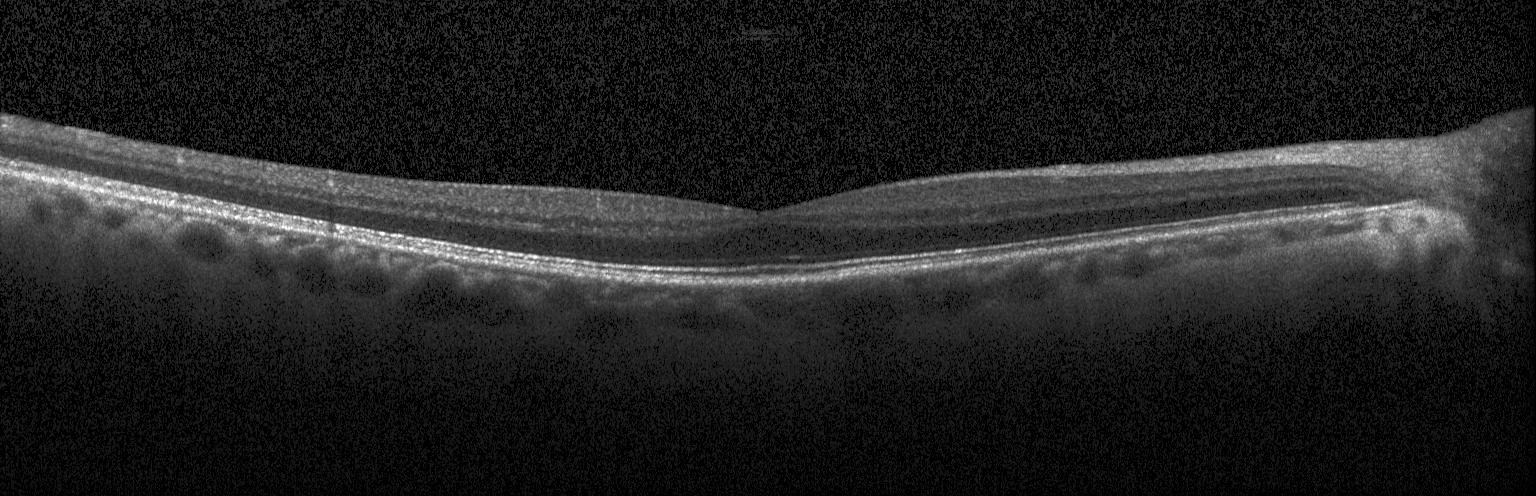

Macular OCT demonstrating no choroidal neovascularization, diabetic macular edema, or drusen.